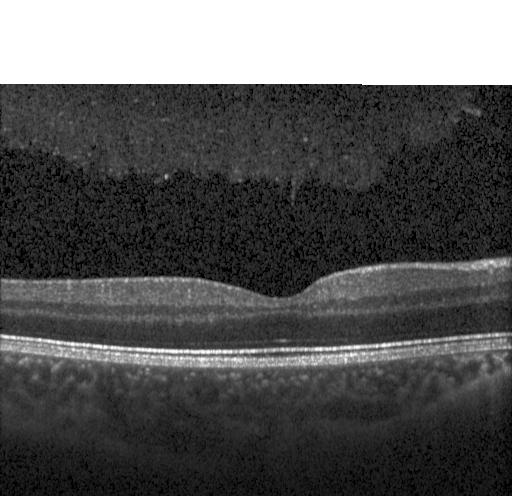 SD-OCT, Heidelberg Spectralis OCT system, OCT B-scan, horizontal scan through the fovea — Diagnosis: neither choroidal neovascularization, diabetic macular edema, nor drusen.